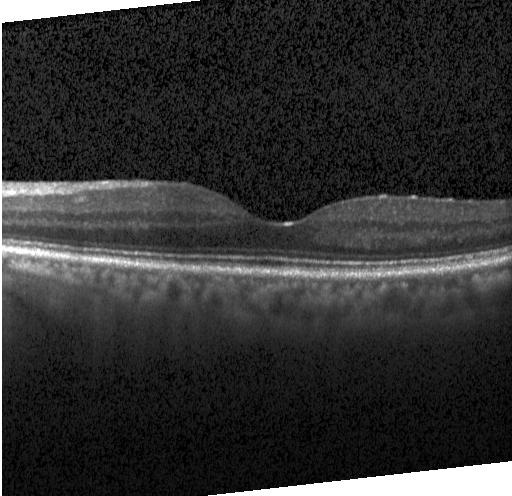

Retinal OCT cross-section — OCT finding: no choroidal neovascularization, no diabetic macular edema, and no drusen.